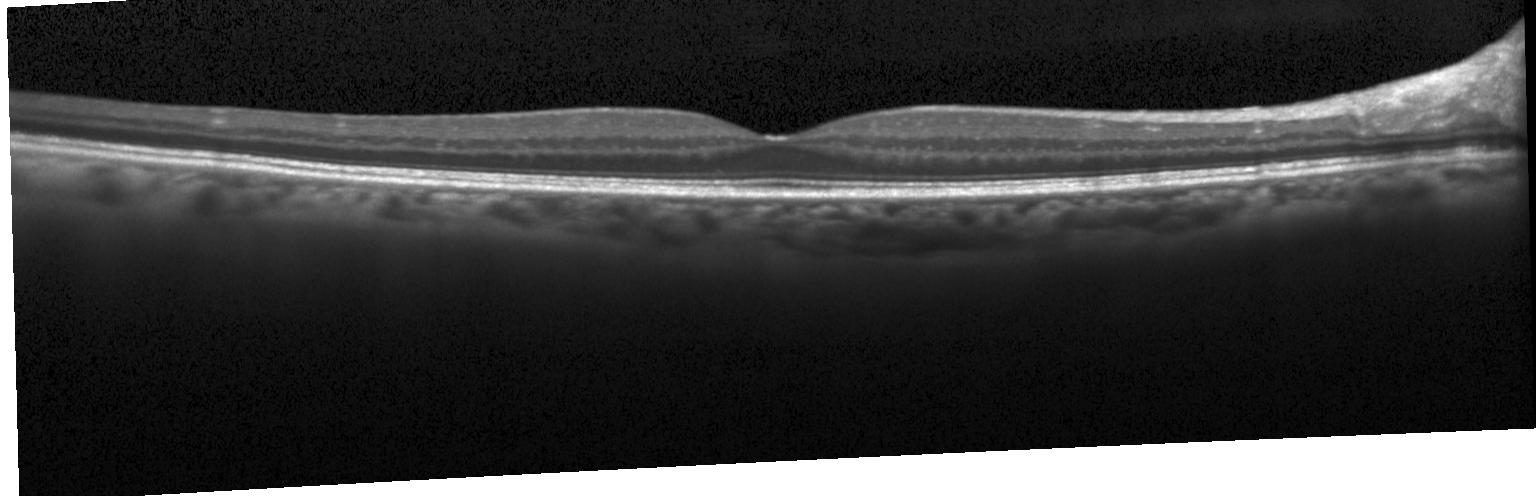 Optical coherence tomography scan. Heidelberg Spectralis. Spectral-domain OCT. Through the macula
This B-scan demonstrates neither CNV, DME, nor drusen.